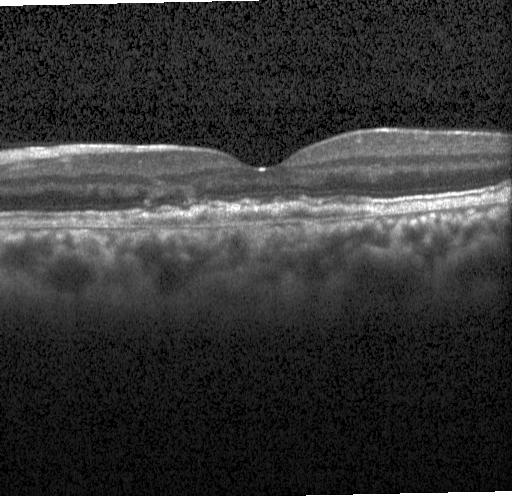

Spectral-domain optical coherence tomography, macular scan, optical coherence tomography scan, Heidelberg Spectralis — OCT finding: CNV.